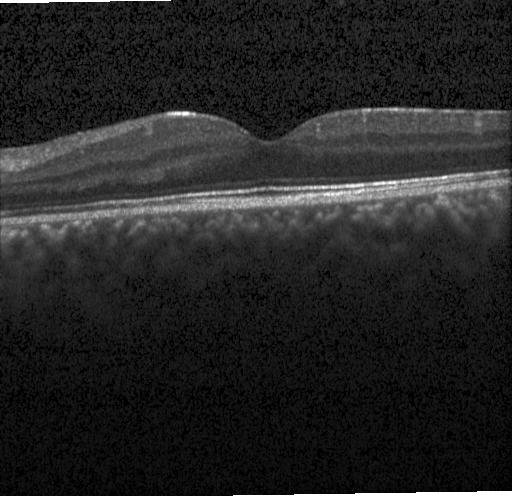
No CNV, no DME, and no drusen.